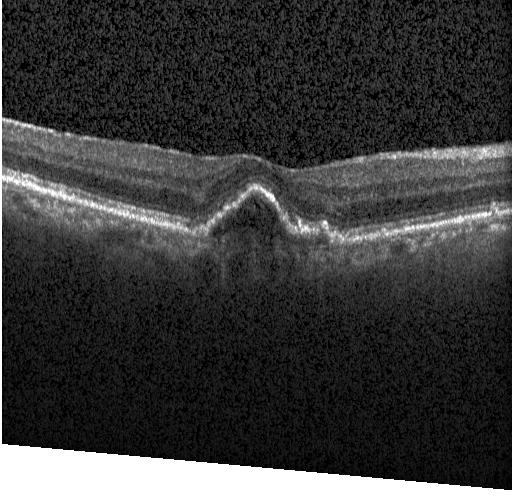 Acquired on a Heidelberg Spectralis, optical coherence tomography scan, spectral-domain OCT — Finding: a choroidal neovascular membrane.